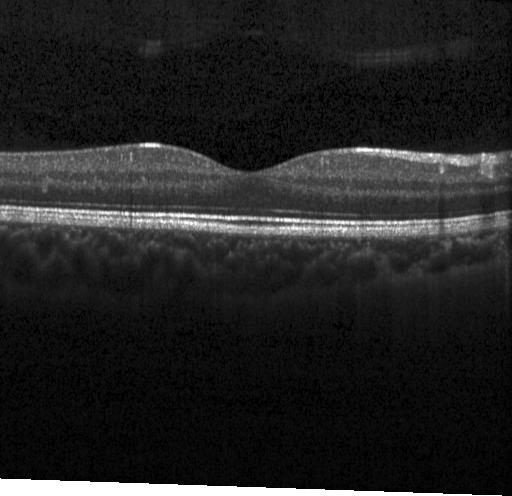 Dx: no choroidal neovascularization, no diabetic macular edema, and no drusen.